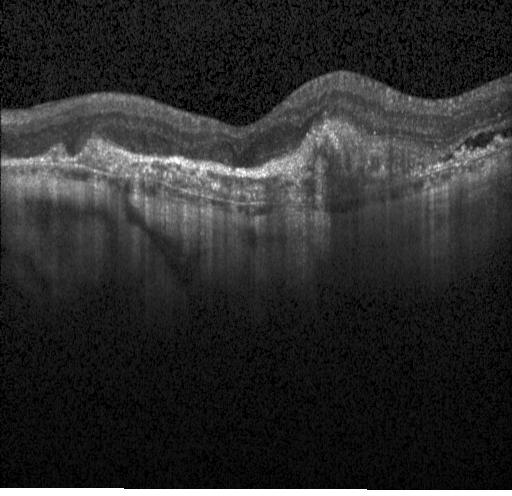 Impression: choroidal neovascularization (CNV).